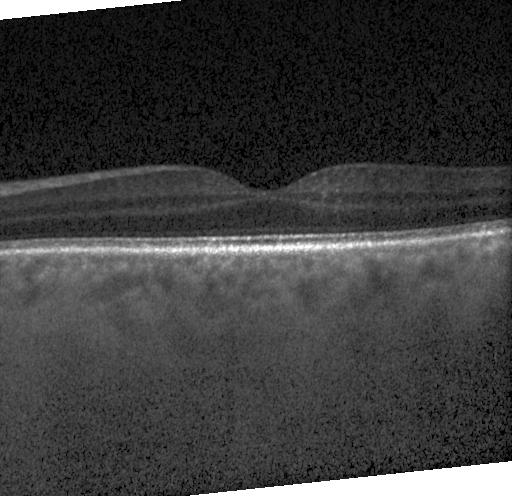

Acquired on a Heidelberg Spectralis. Retinal OCT cross-section. Fovea-centered
OCT finding: no CNV, DME, or drusen.